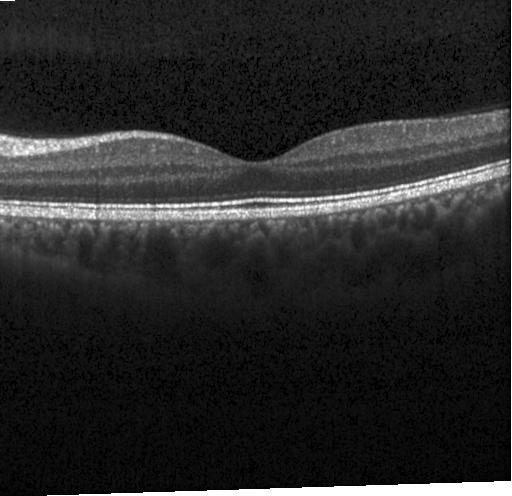
Spectral-domain OCT. Retinal OCT cross-section. Heidelberg Spectralis OCT system.
Impression: no evidence of choroidal neovascularization, diabetic macular edema, or drusen.